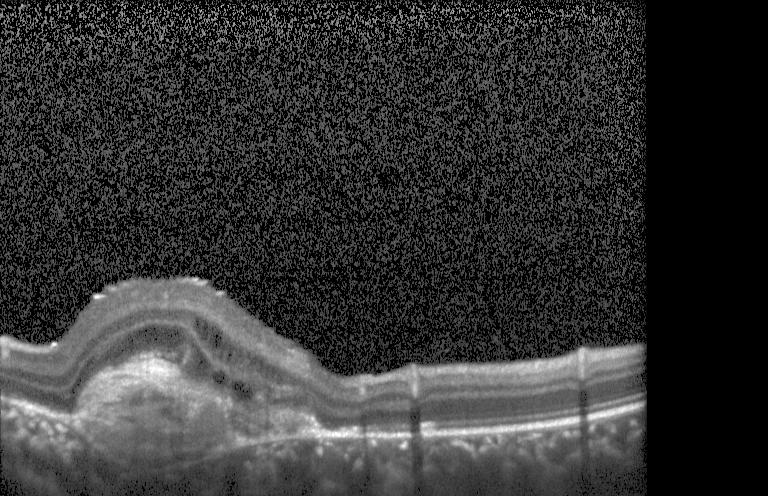

CNV.